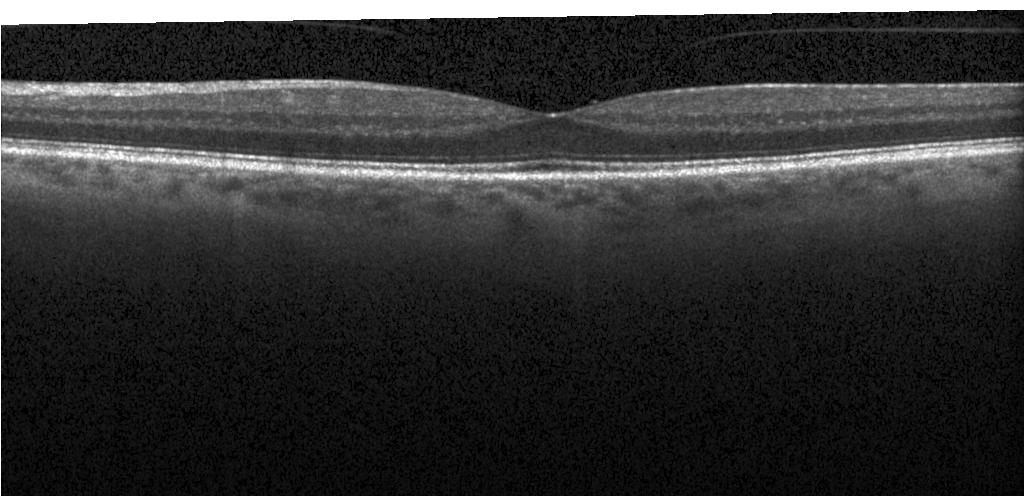

OCT line scan; Heidelberg Spectralis OCT system; centered on the fovea — This B-scan demonstrates neither choroidal neovascularization, diabetic macular edema, nor drusen.